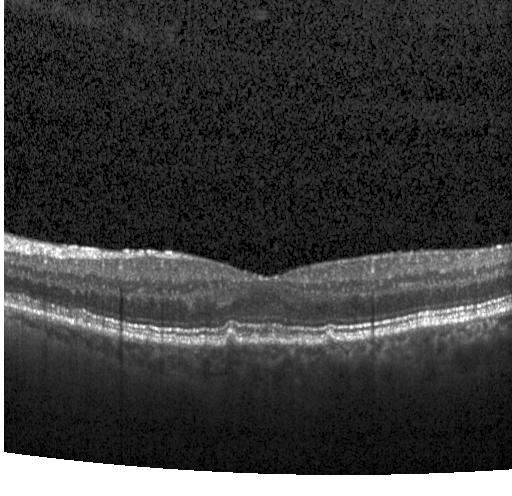
Diagnosis: multiple drusen.